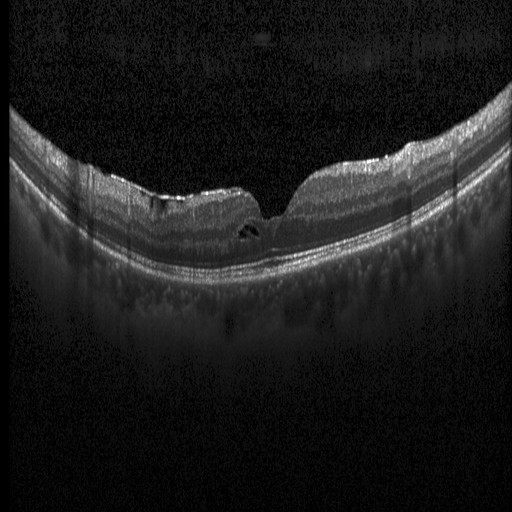

Retinal OCT B-scan. SD-OCT. Heidelberg Spectralis. Through the macula
DME.